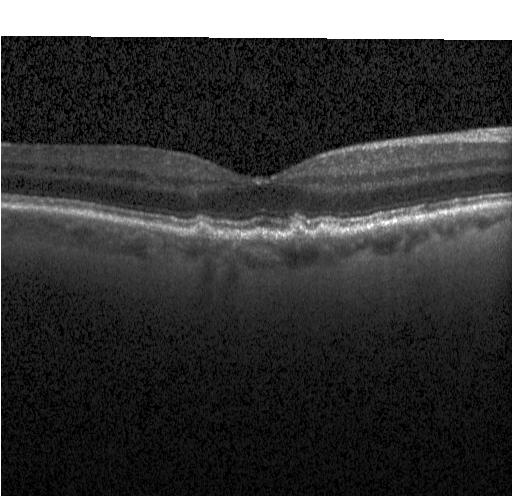

OCT B-scan
Diagnosis: multiple drusen.